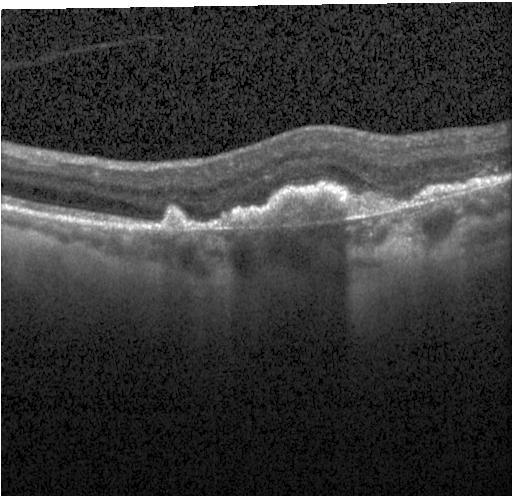

The scan shows a choroidal neovascular membrane.